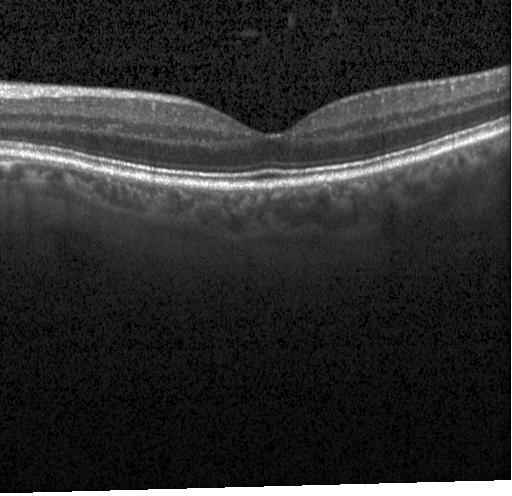 Spectral-domain OCT, OCT B-scan, Heidelberg Spectralis OCT system. No CNV, DME, or drusen.